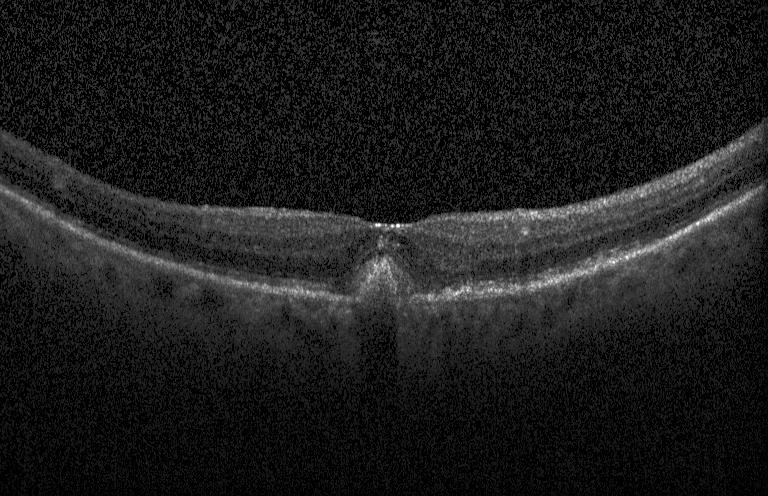

Optical coherence tomography B-scan — Diagnosis: a choroidal neovascular membrane.